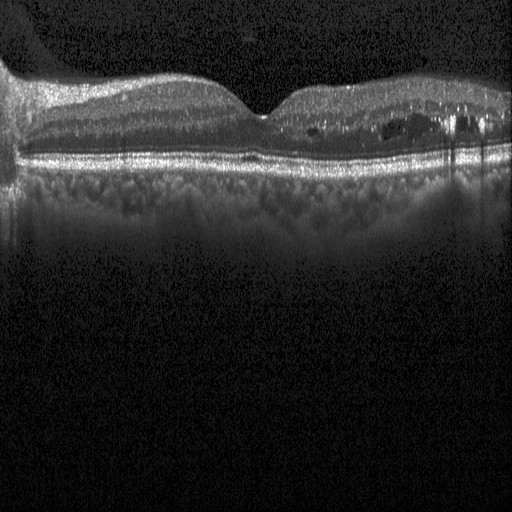

Retinal OCT B-scan, Heidelberg Spectralis — Finding: diabetic macular edema.